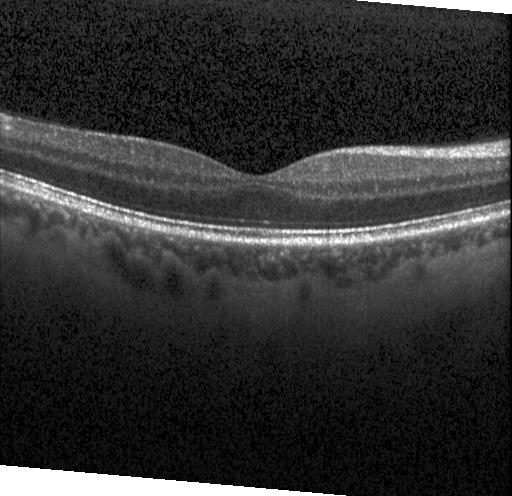
Heidelberg Spectralis OCT system · optical coherence tomography scan · through the macula — Finding: no choroidal neovascularization, diabetic macular edema, or drusen.